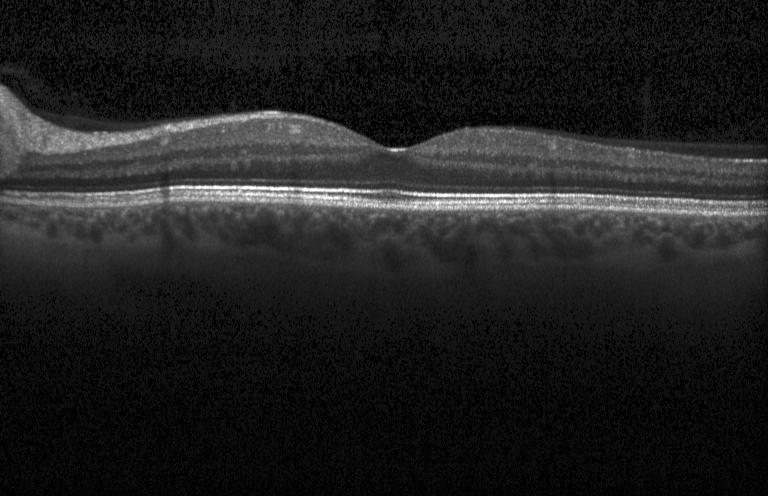 Spectral-domain OCT B-scan: no evidence of CNV, DME, or drusen.